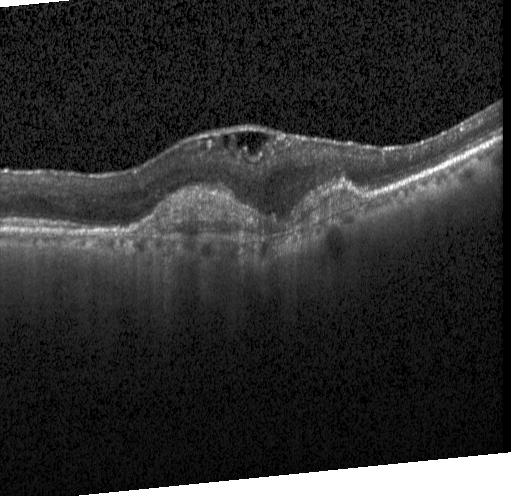
Finding: choroidal neovascularization (CNV).